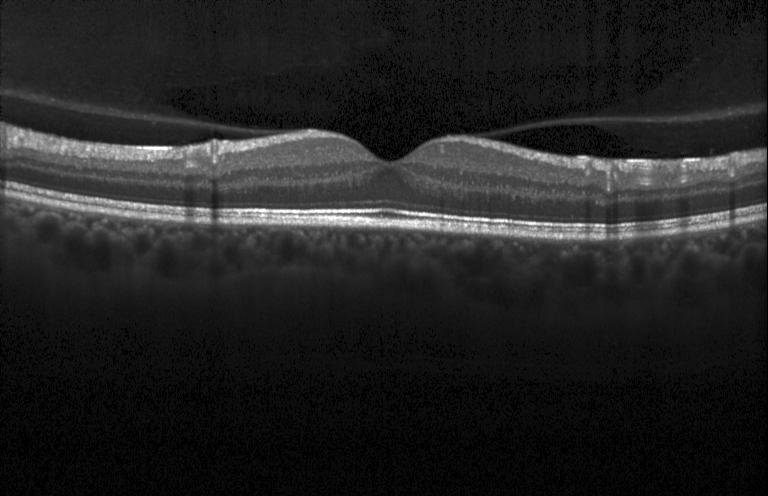 Finding: neither choroidal neovascularization, diabetic macular edema, nor drusen.